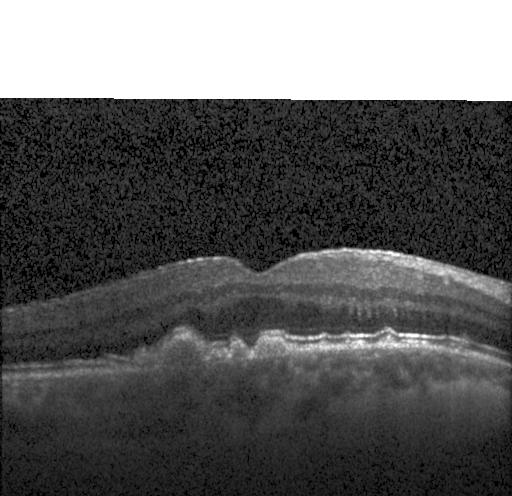
OCT B-scan showing multiple drusen.